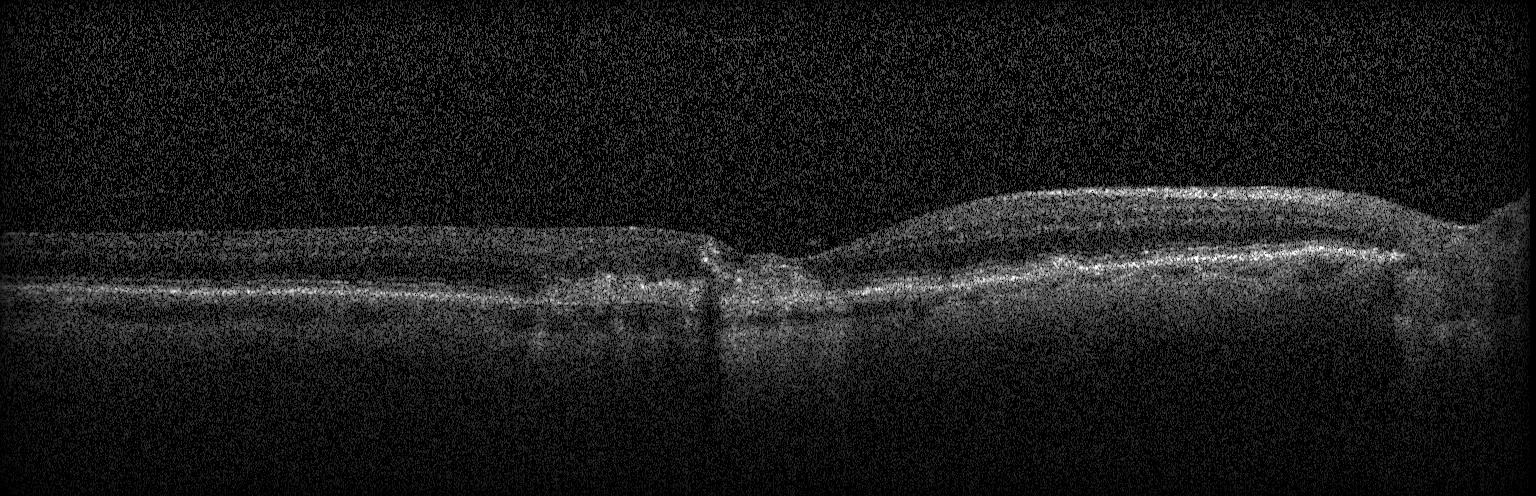
OCT line scan.
Diagnosis: choroidal neovascularization (CNV).